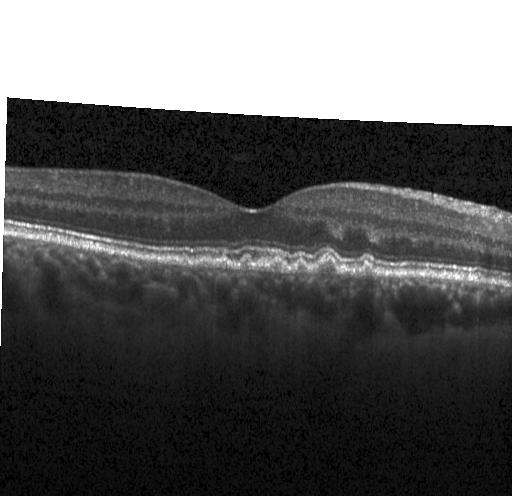 Retinal OCT B-scan. Impression: multiple drusen.